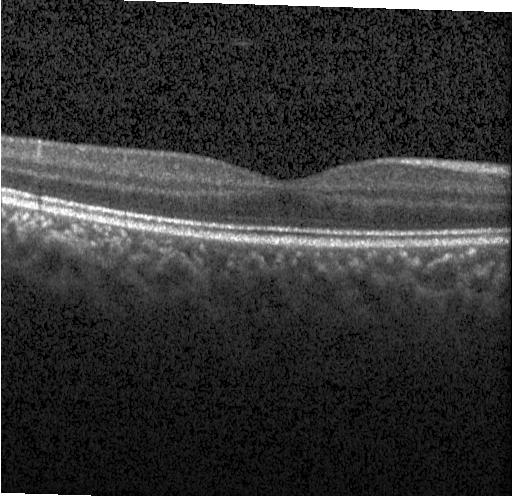
Retinal OCT cross-section. This B-scan demonstrates no choroidal neovascularization, diabetic macular edema, or drusen.